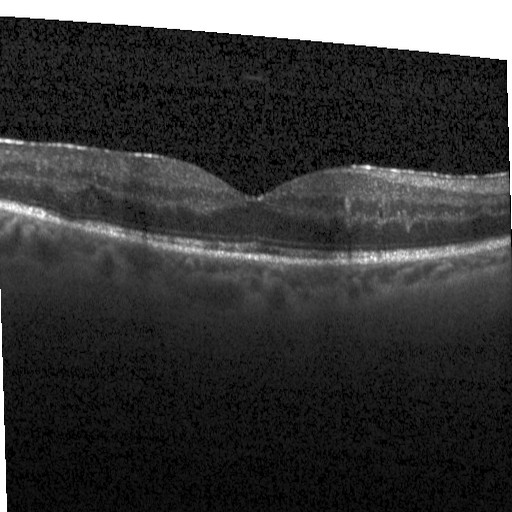

Dx: DME.